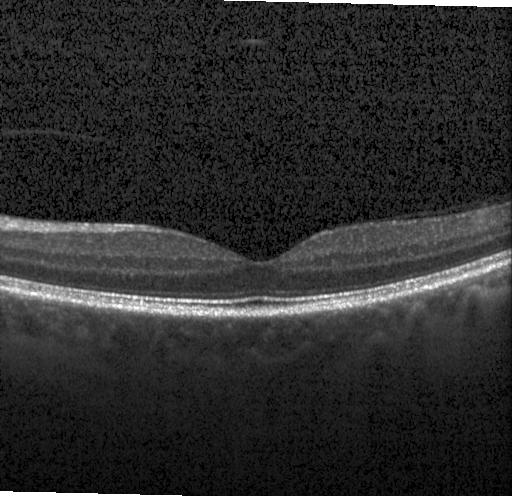 OCT B-scan
Impression: no CNV, no DME, and no drusen.